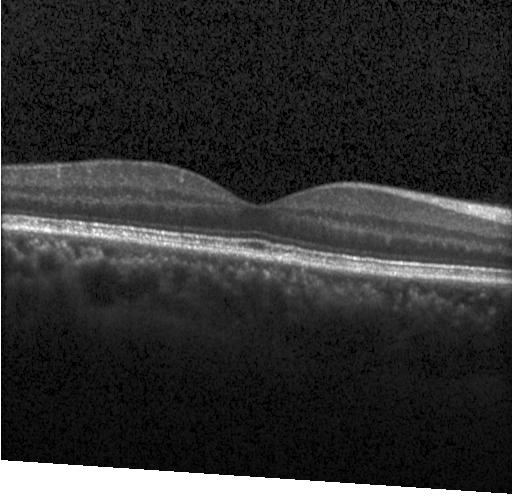

Centered on the fovea · spectral-domain optical coherence tomography · optical coherence tomography scan · Heidelberg Spectralis — Impression: no evidence of choroidal neovascularization, diabetic macular edema, or drusen.